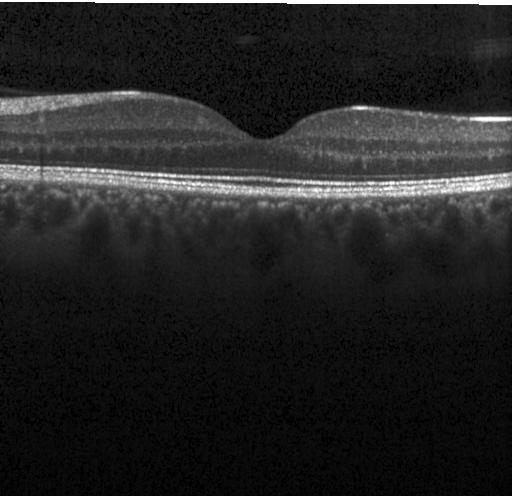 Macular OCT demonstrating no evidence of choroidal neovascularization, diabetic macular edema, or drusen.